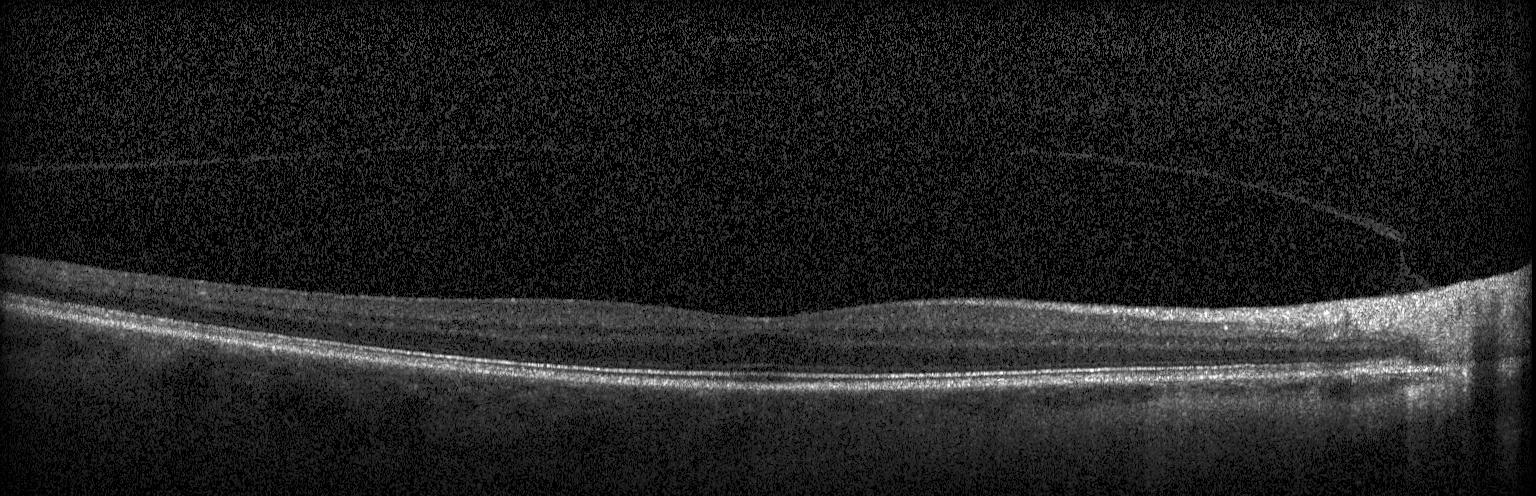
Assessment: neither CNV, DME, nor drusen.